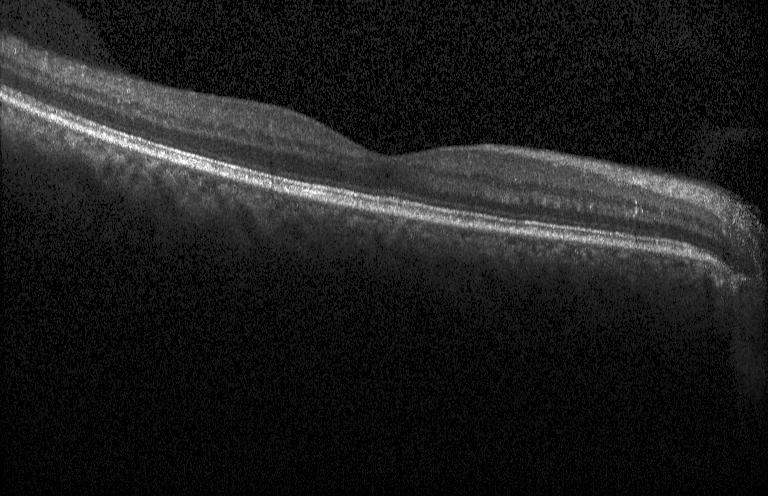

Acquired on a Heidelberg Spectralis, OCT B-scan
Impression: no choroidal neovascularization, diabetic macular edema, or drusen.